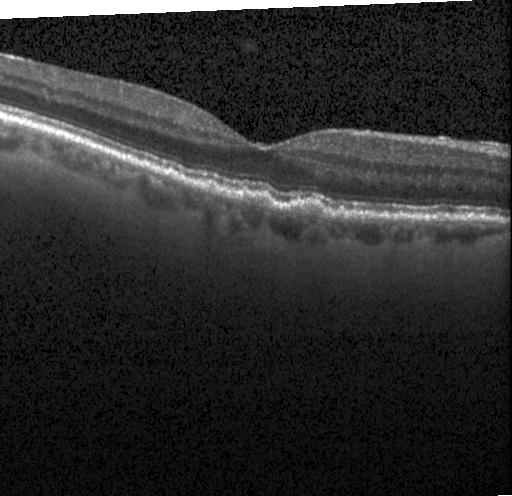 Acquired on a Heidelberg Spectralis; fovea-centered; OCT line scan
Macular OCT: sub-RPE drusenoid deposits.